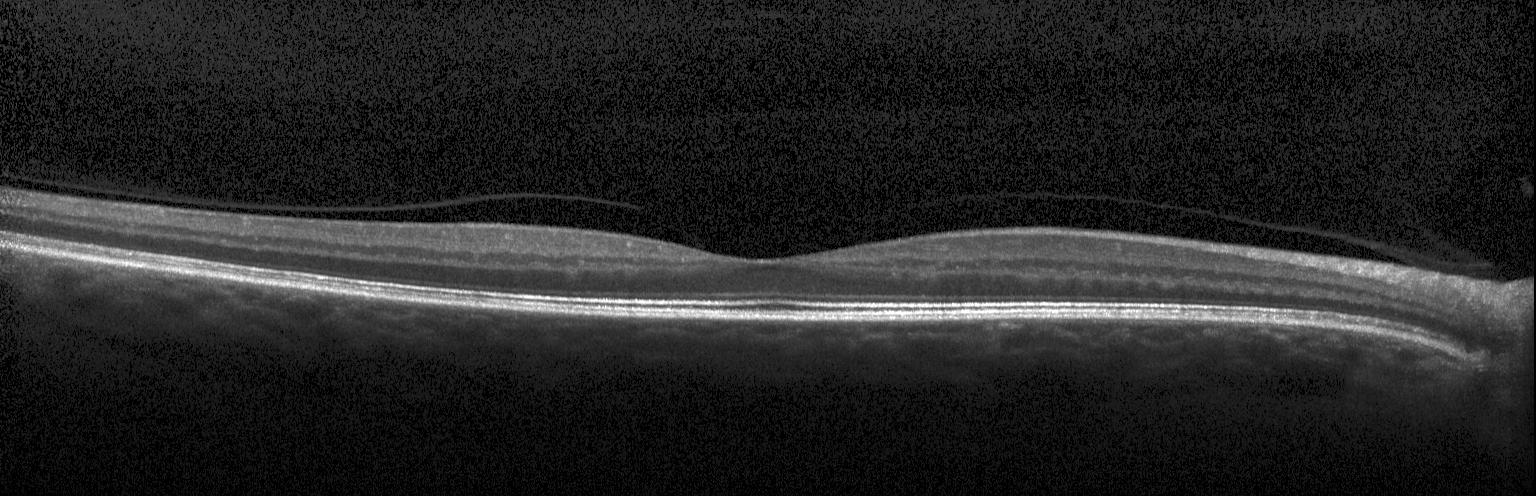 Impression: no CNV, no DME, and no drusen.